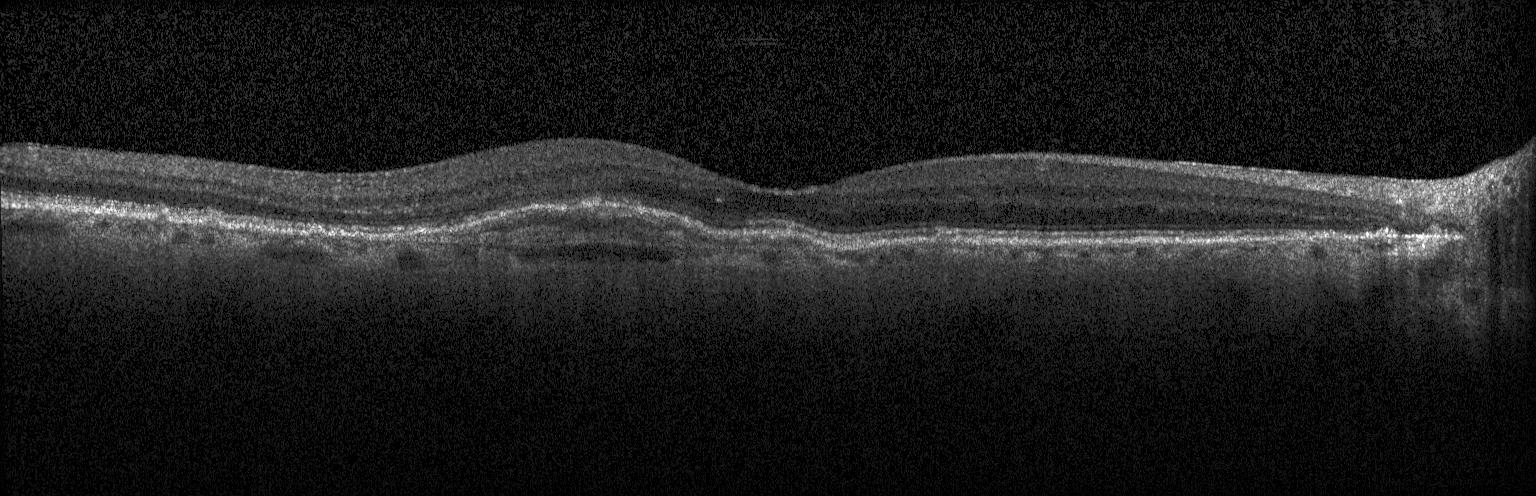
Fovea-centered, retinal OCT B-scan. Macular OCT: choroidal neovascularization.